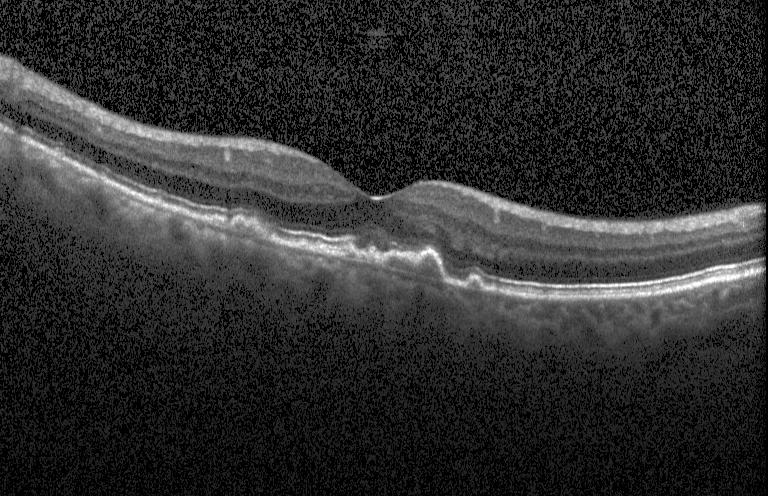 Macular OCT demonstrating sub-RPE drusenoid deposits.